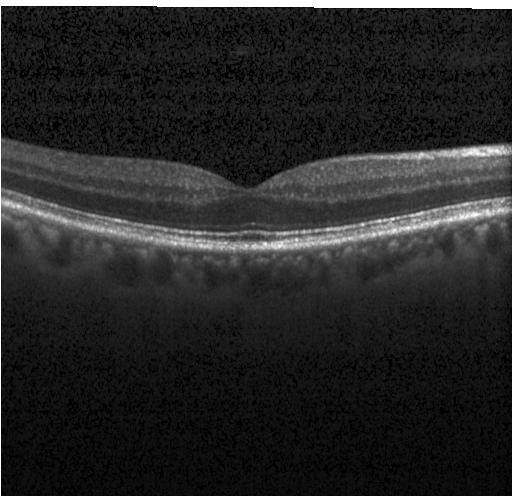
This B-scan demonstrates no choroidal neovascularization, no diabetic macular edema, and no drusen.